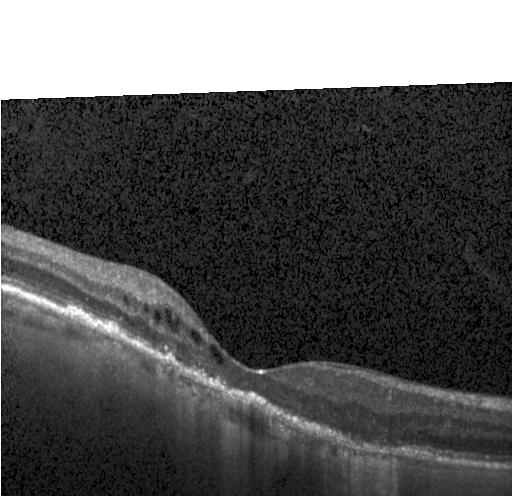

OCT B-scan showing choroidal neovascularization.